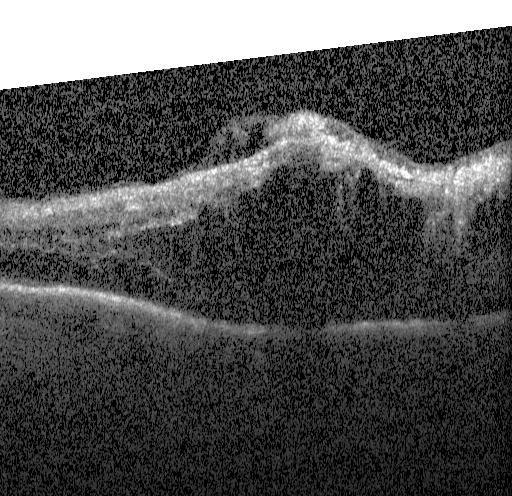

Impression: diabetic macular edema.